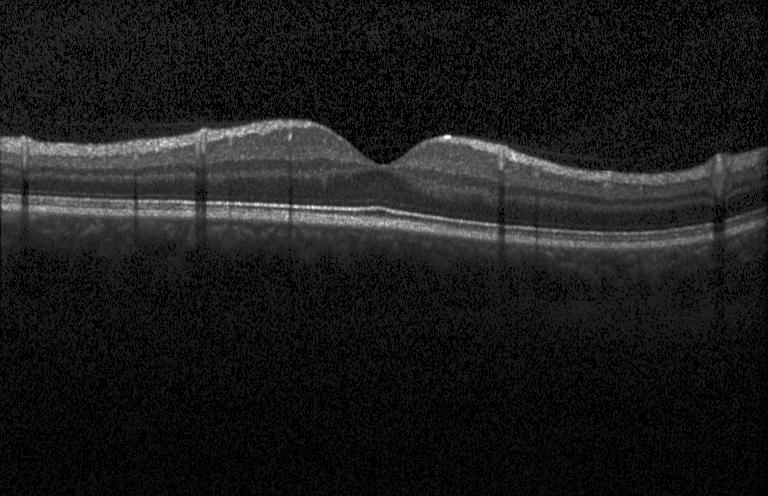 Retinal OCT cross-section; Heidelberg Spectralis — No evidence of CNV, DME, or drusen.